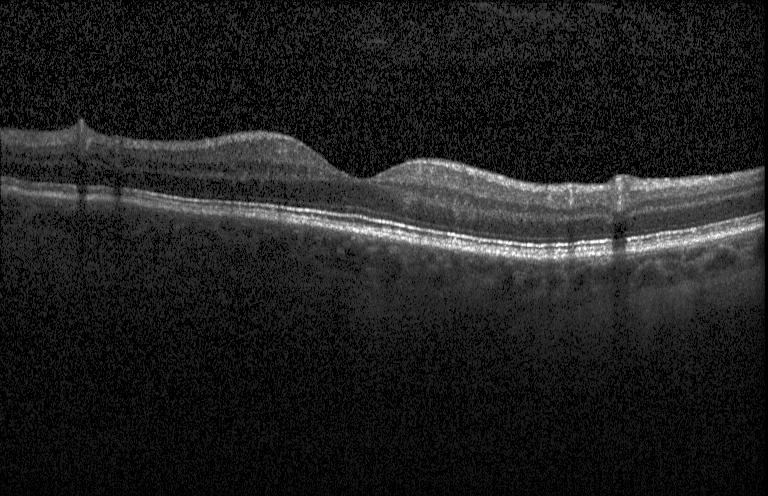 OCT B-scan showing no choroidal neovascularization, diabetic macular edema, or drusen.